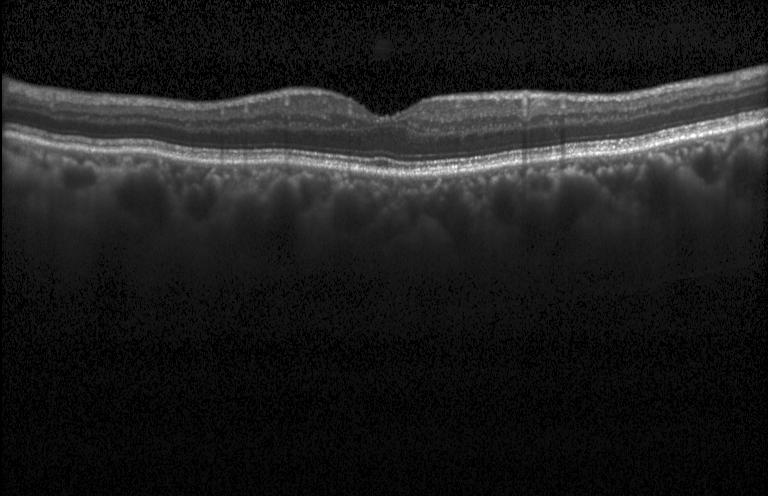

Spectral-domain OCT, retinal OCT cross-section. Finding: no choroidal neovascularization, no diabetic macular edema, and no drusen.